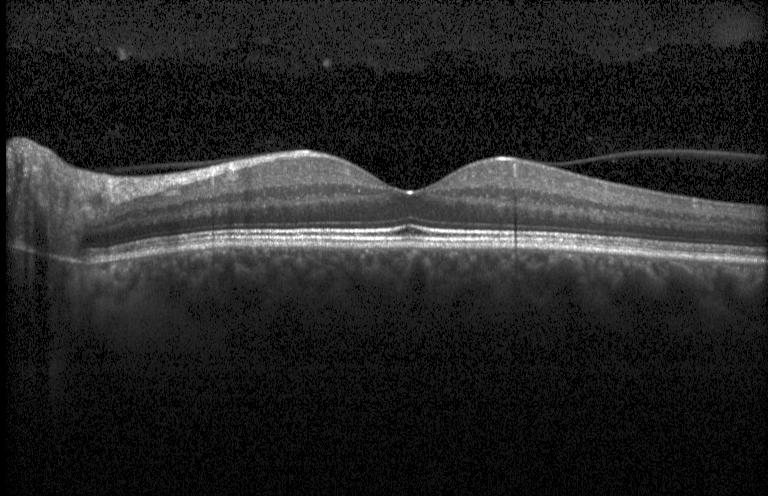

Assessment: no evidence of CNV, DME, or drusen.